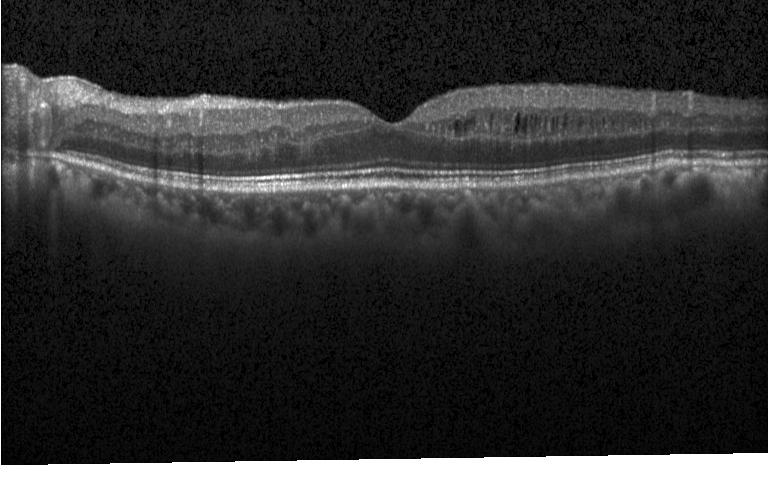

OCT B-scan showing diabetic macular edema (DME).